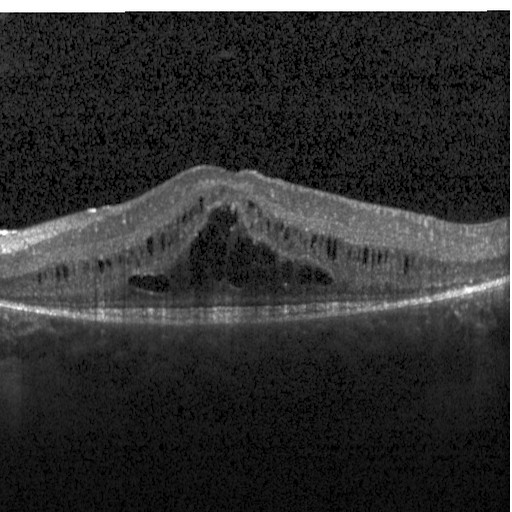
Macular OCT demonstrating DME.